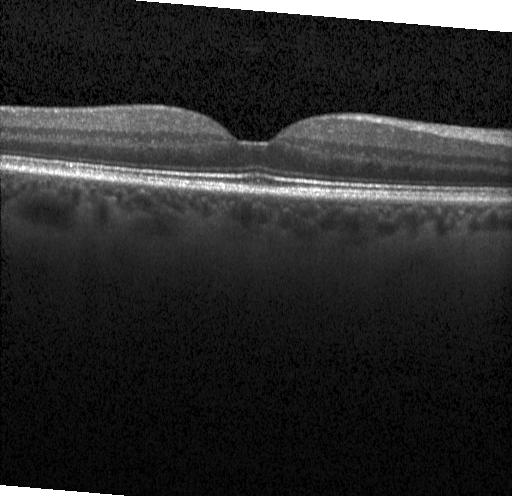 This B-scan demonstrates no evidence of choroidal neovascularization, diabetic macular edema, or drusen.